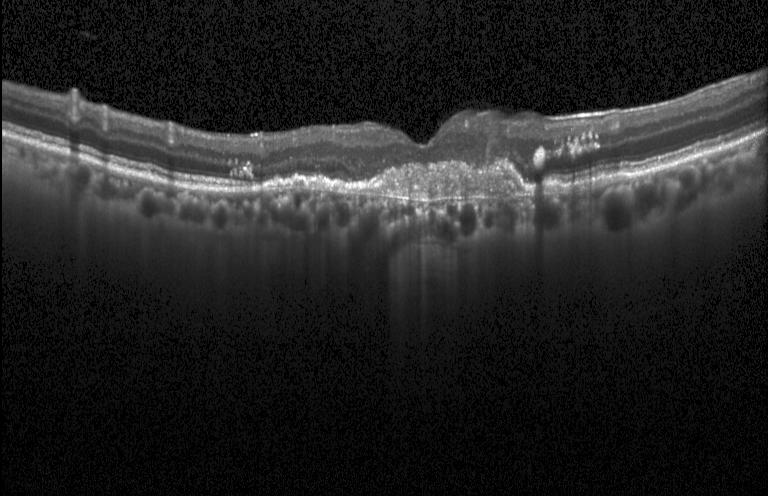

Spectral-domain OCT; optical coherence tomography B-scan.
Impression: a choroidal neovascular membrane.